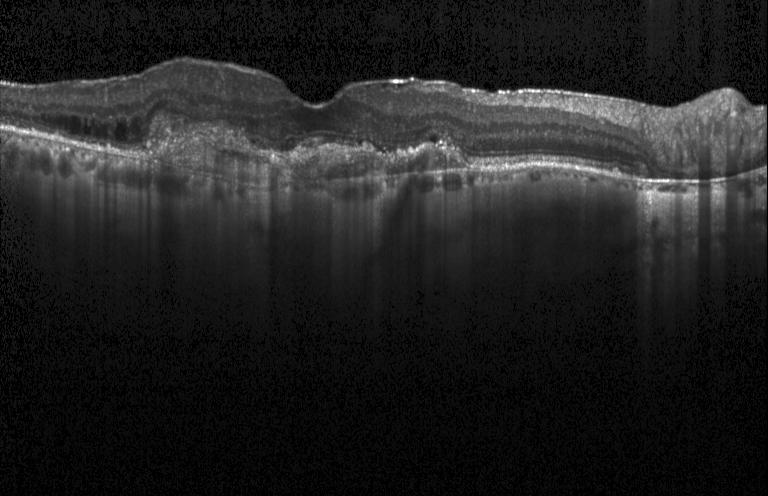

A choroidal neovascular membrane.